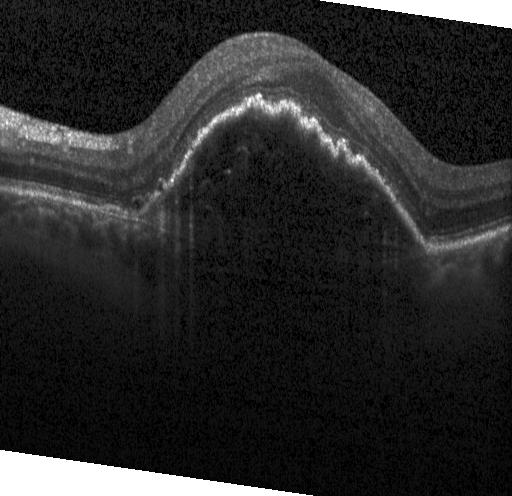 OCT line scan. Heidelberg Spectralis. Fovea-centered. Spectral-domain OCT — Diagnosis: a choroidal neovascular membrane.